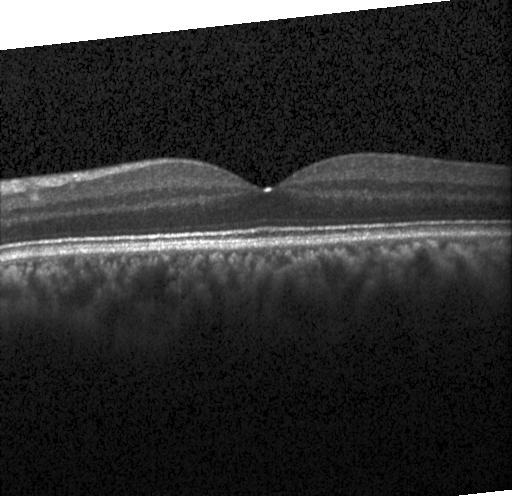

OCT scan showing no CNV, DME, or drusen.